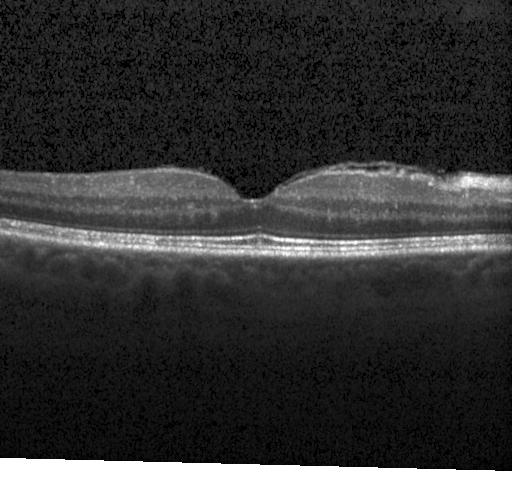 Finding: no evidence of choroidal neovascularization, diabetic macular edema, or drusen.